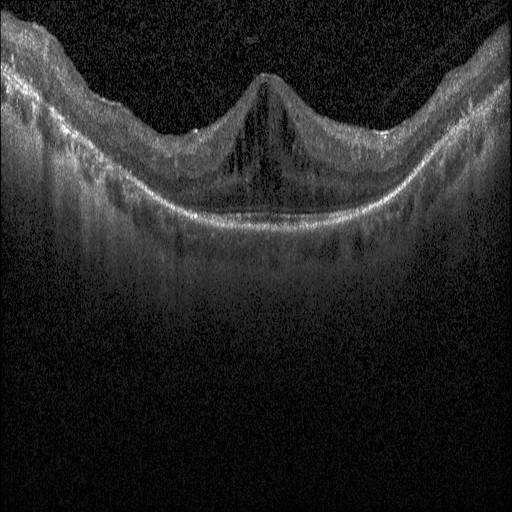 Optical coherence tomography B-scan; instrument: Heidelberg Spectralis; spectral-domain OCT. Finding: diabetic macular edema (DME).